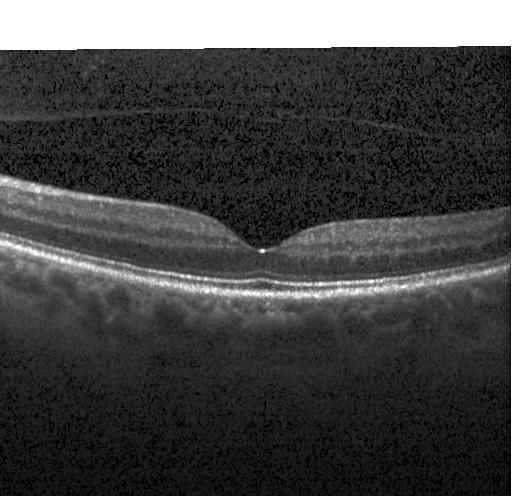
Optical coherence tomography scan · SD-OCT
This B-scan demonstrates no evidence of CNV, DME, or drusen.